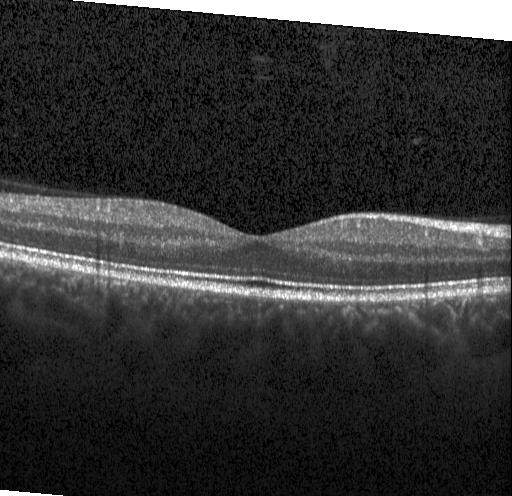 Centered on the fovea, spectral-domain optical coherence tomography, instrument: Heidelberg Spectralis, optical coherence tomography B-scan
The scan shows neither choroidal neovascularization, diabetic macular edema, nor drusen.